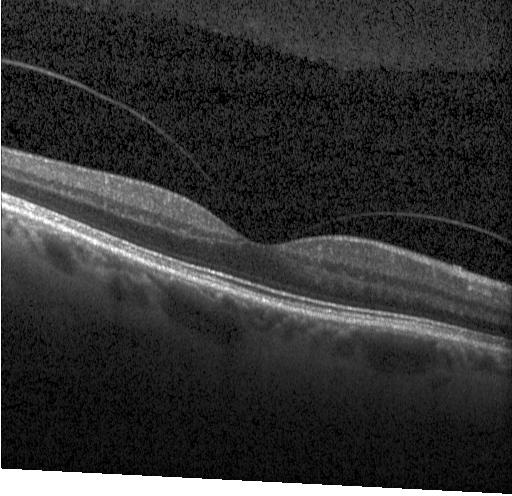 Optical coherence tomography scan — Assessment: no choroidal neovascularization, diabetic macular edema, or drusen.